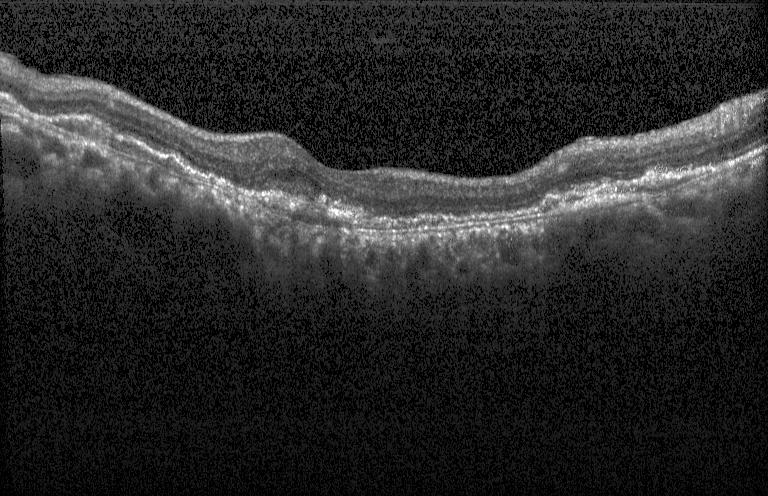 Optical coherence tomography scan · SD-OCT · through the macula.
Finding: a choroidal neovascular membrane.